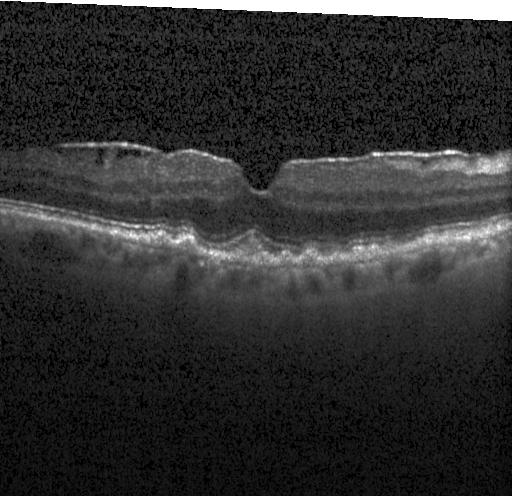 Impression: sub-RPE drusenoid deposits.